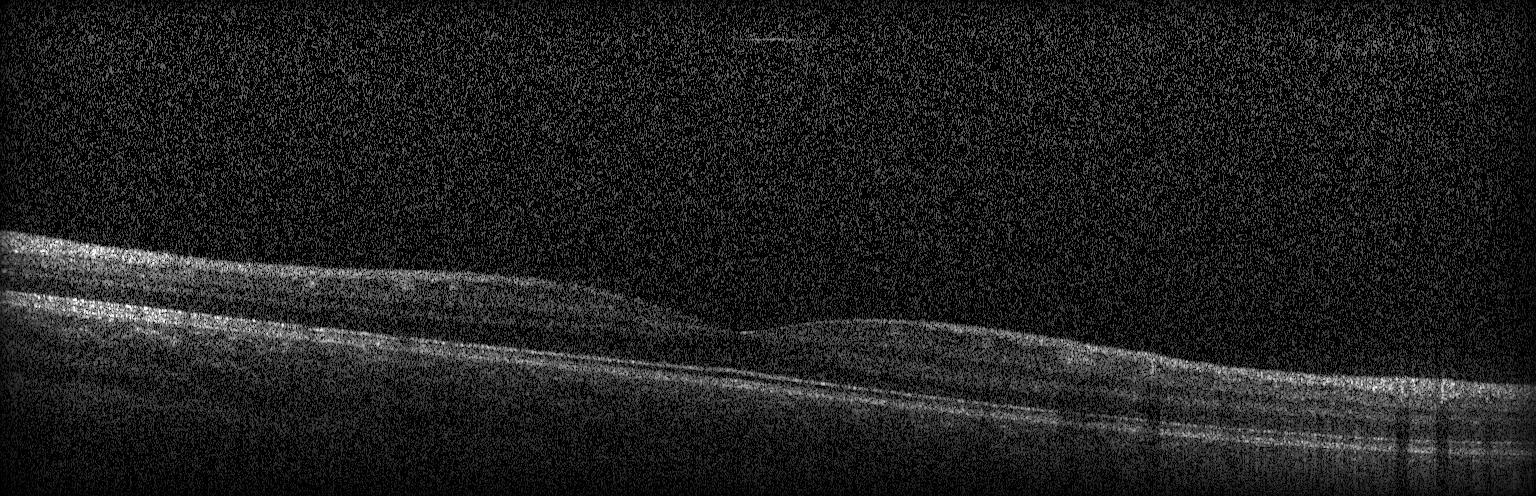

Retinal OCT cross-section. No choroidal neovascularization, no diabetic macular edema, and no drusen.